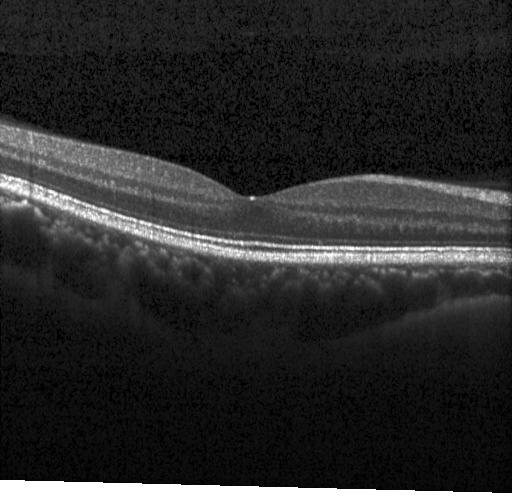
Spectral-domain optical coherence tomography · horizontal scan through the fovea · retinal OCT B-scan · instrument: Heidelberg Spectralis. Finding: neither choroidal neovascularization, diabetic macular edema, nor drusen.